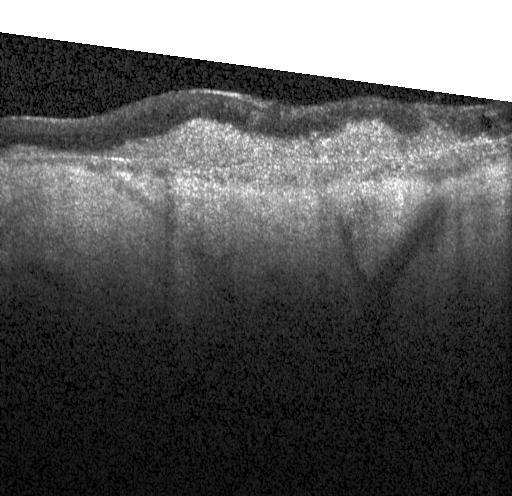
Acquired on a Heidelberg Spectralis, retinal OCT B-scan, spectral-domain optical coherence tomography, fovea-centered — Finding: a choroidal neovascular membrane.